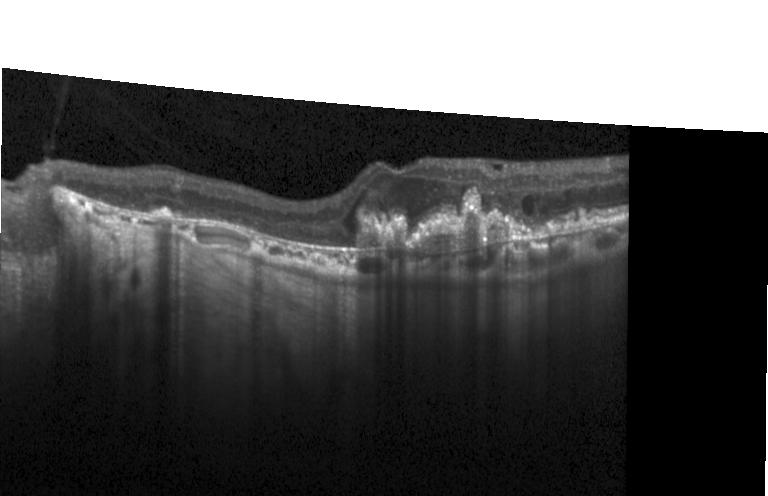 SD-OCT · retinal OCT cross-section · acquired on a Heidelberg Spectralis
Finding: a choroidal neovascular membrane.